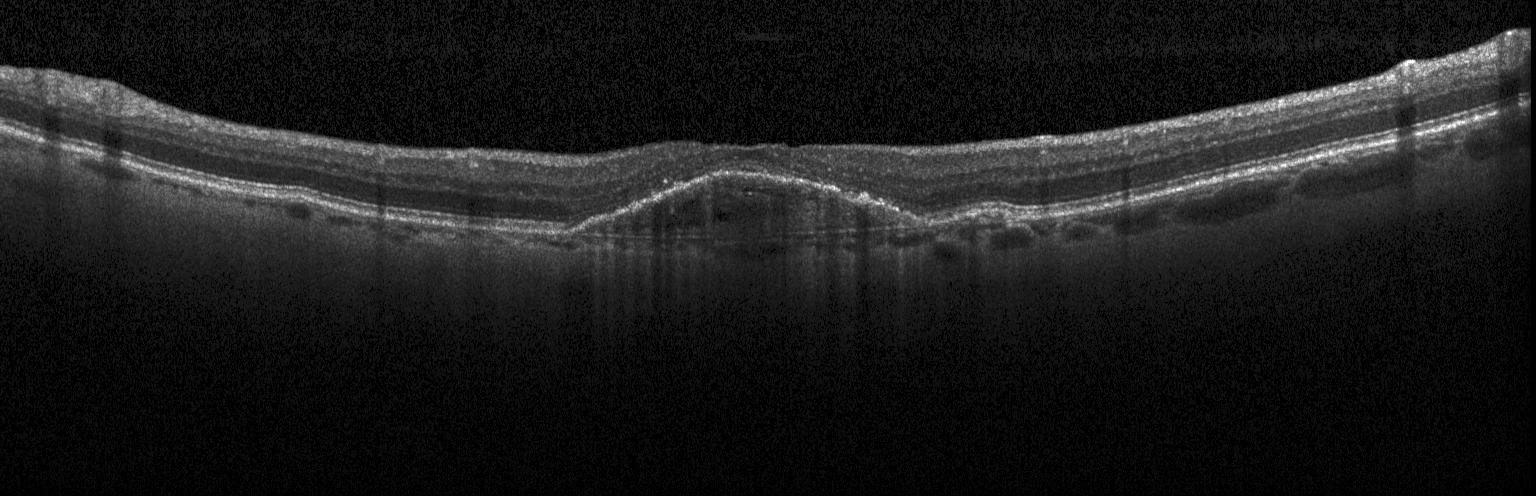 OCT scan showing a choroidal neovascular membrane.